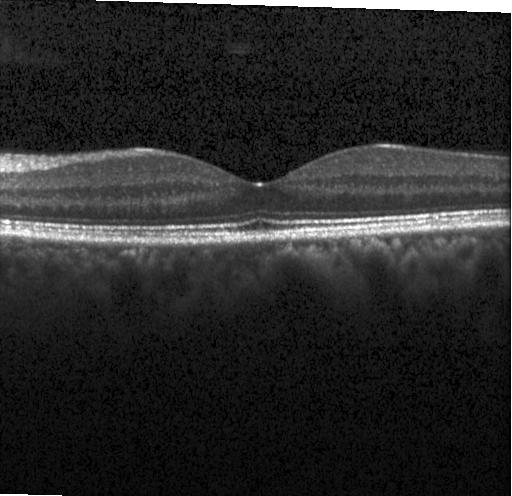
Macular OCT demonstrating no CNV, no DME, and no drusen.